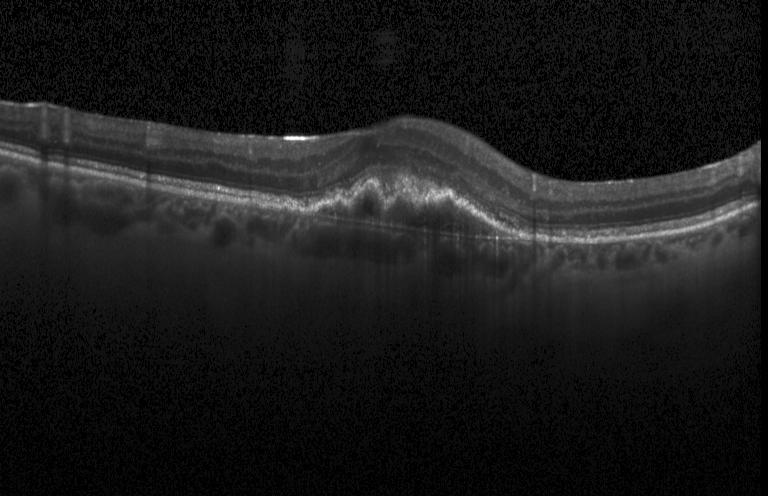 Optical coherence tomography B-scan.
Macular OCT: a choroidal neovascular membrane.